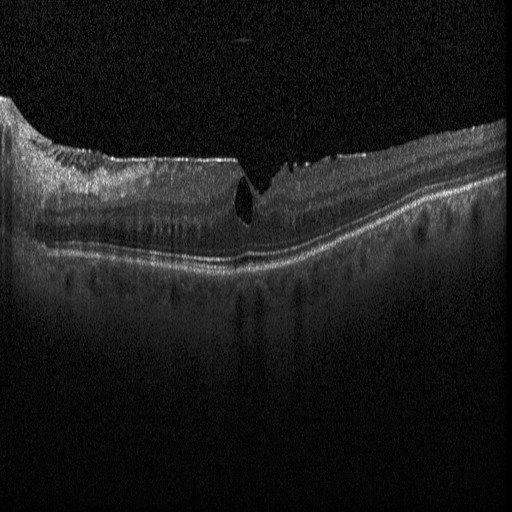

The scan shows diabetic macular edema.